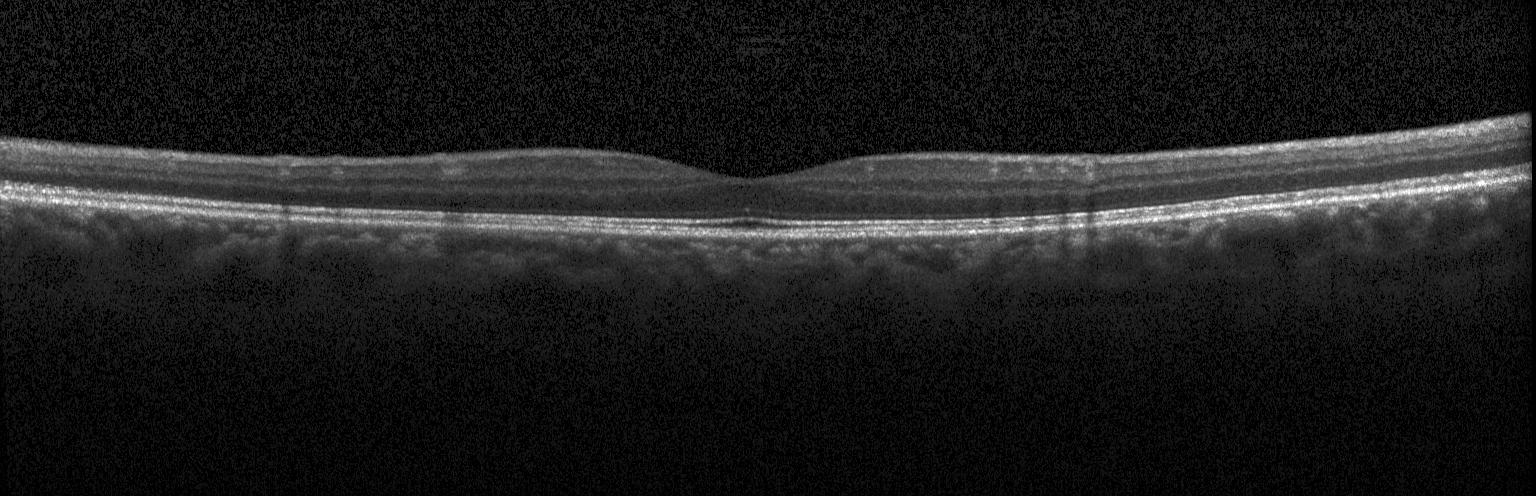 Assessment: no choroidal neovascularization, no diabetic macular edema, and no drusen.